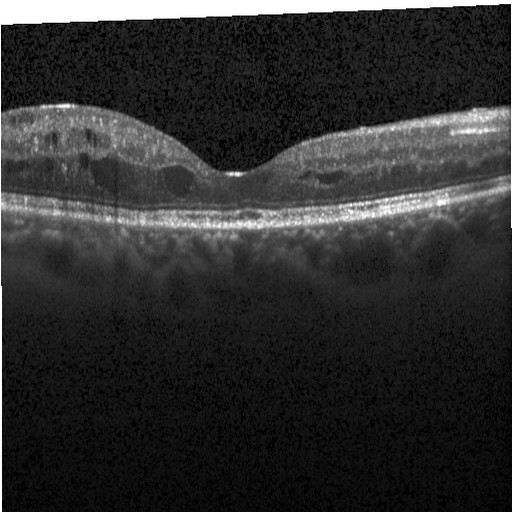 Finding: DME.